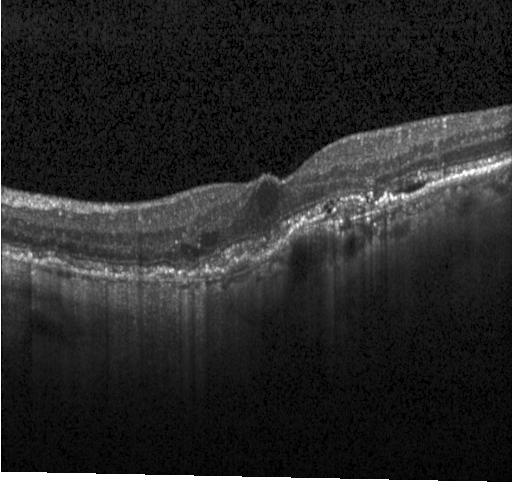

Horizontal scan through the fovea. Retinal OCT B-scan. Impression: choroidal neovascularization.